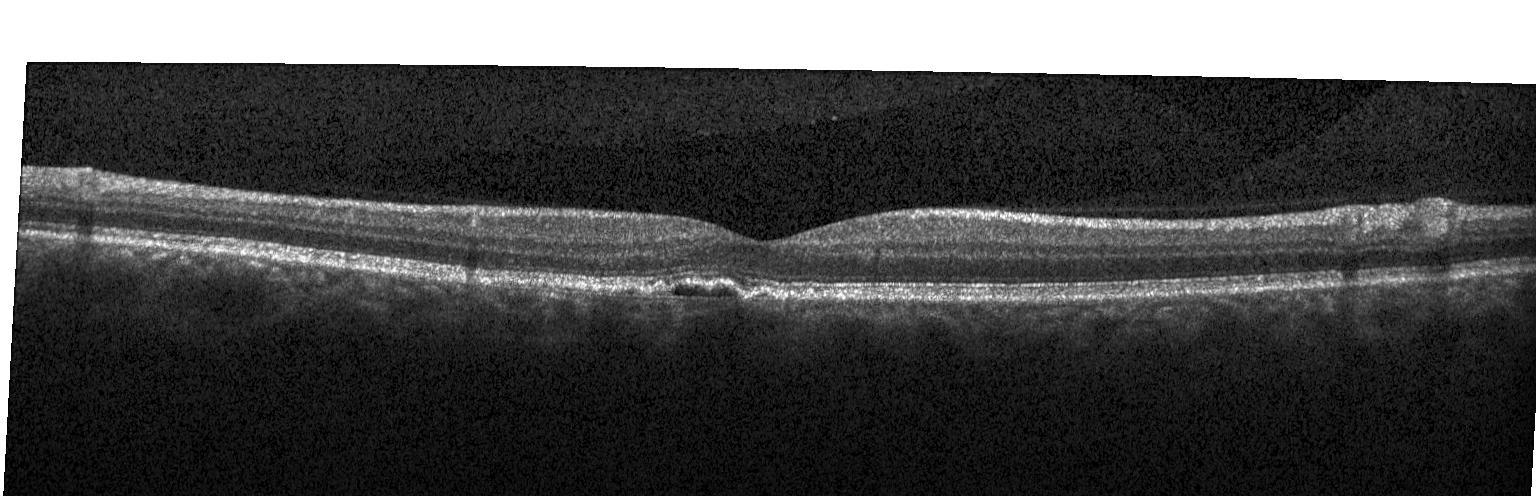 Instrument: Heidelberg Spectralis. Spectral-domain optical coherence tomography. Optical coherence tomography B-scan.
Impression: choroidal neovascularization (CNV).